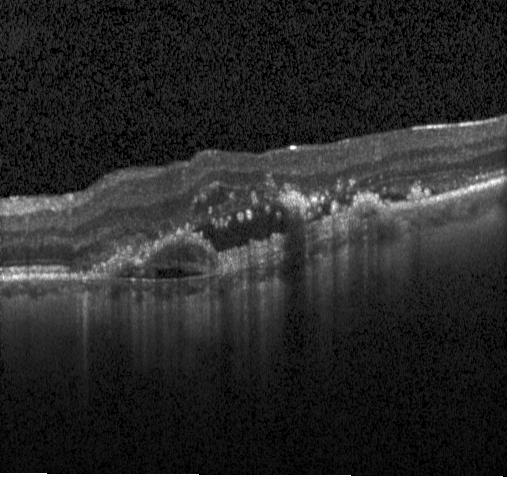
Optical coherence tomography B-scan; spectral-domain OCT; Heidelberg Spectralis
Macular OCT: choroidal neovascularization.